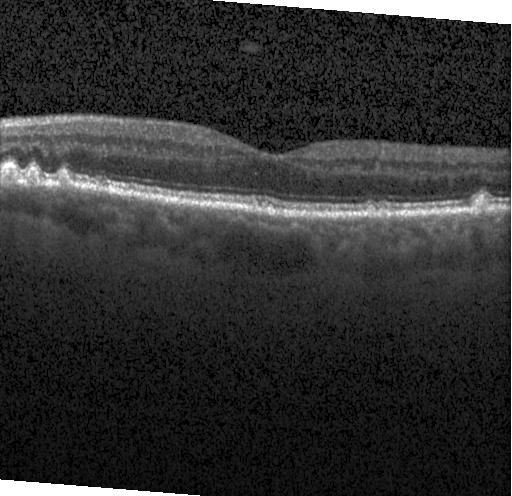 OCT line scan; horizontal scan through the fovea; acquired on a Heidelberg Spectralis; spectral-domain optical coherence tomography — Diagnosis: sub-RPE drusenoid deposits.